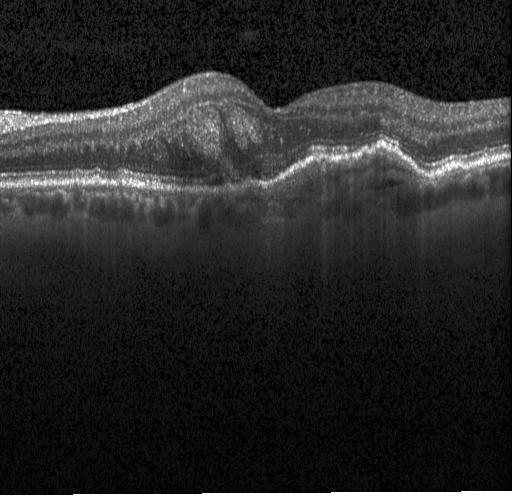
Retinal OCT B-scan, macular scan.
Diagnosis: CNV.